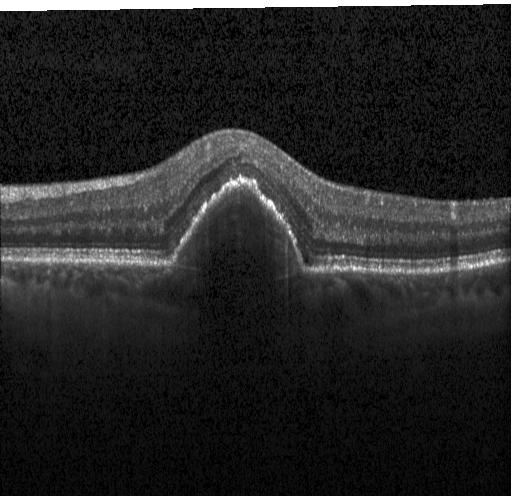

Heidelberg Spectralis; optical coherence tomography B-scan. Diagnosis: a choroidal neovascular membrane.